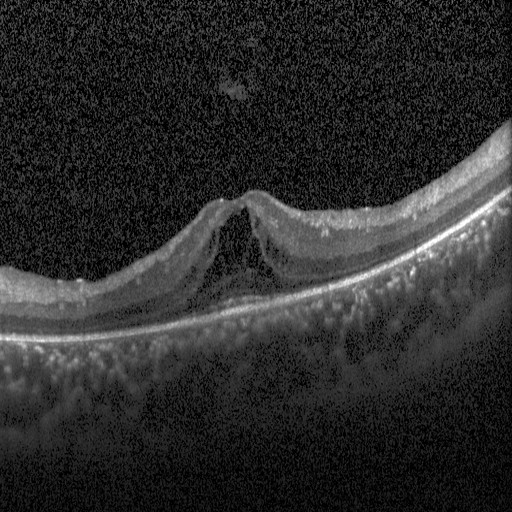
Macular OCT: diabetic macular edema.